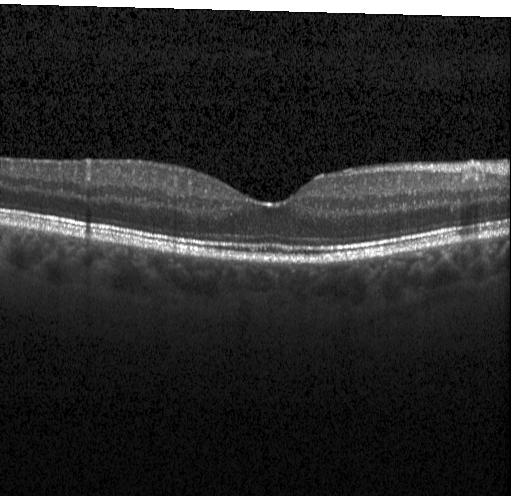

OCT line scan, SD-OCT
Finding: no choroidal neovascularization, no diabetic macular edema, and no drusen.